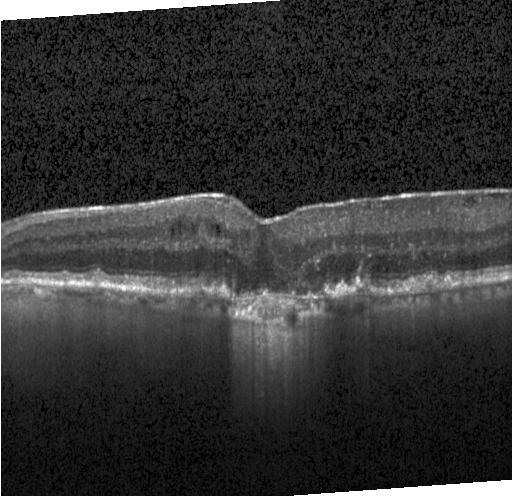

Impression: a choroidal neovascular membrane.